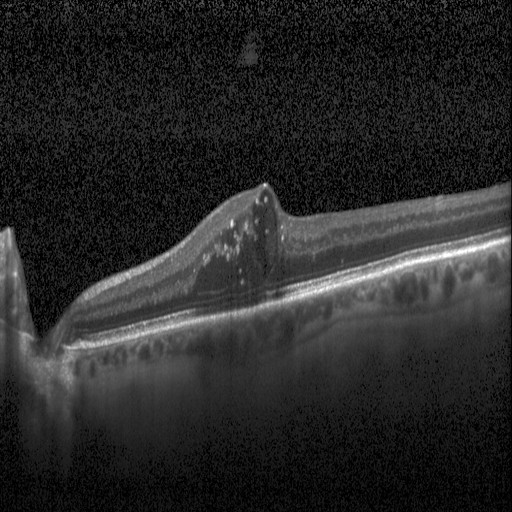
This B-scan demonstrates diabetic macular edema.